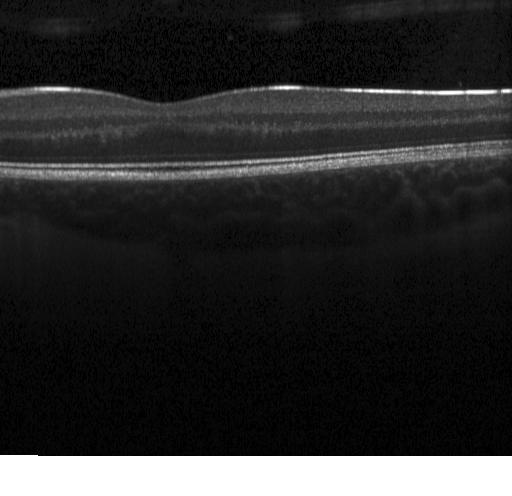
Retinal OCT B-scan; spectral-domain optical coherence tomography; instrument: Heidelberg Spectralis — Assessment: no evidence of CNV, DME, or drusen.